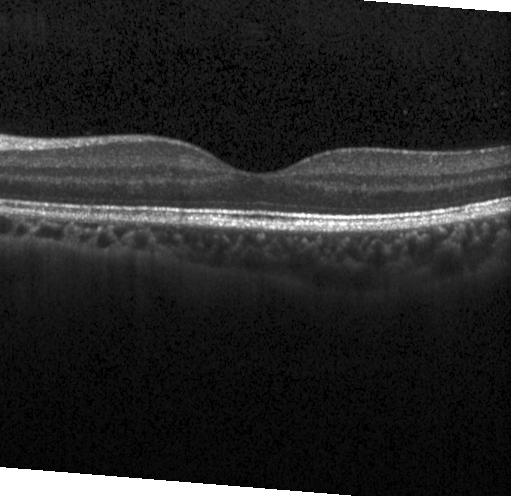

OCT B-scan; Heidelberg Spectralis; fovea-centered
Assessment: no choroidal neovascularization, no diabetic macular edema, and no drusen.